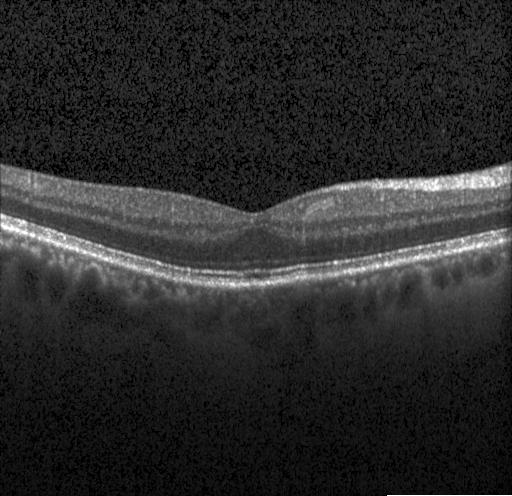
Retinal OCT cross-section. Through the macula
Impression: no evidence of choroidal neovascularization, diabetic macular edema, or drusen.